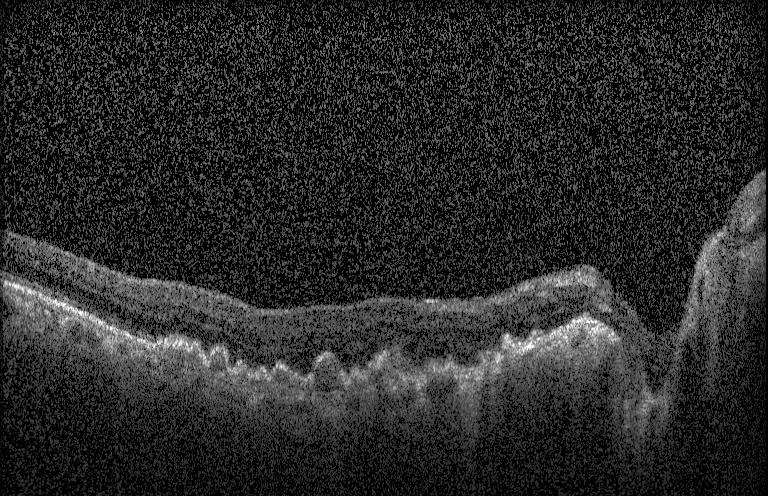

Macular OCT demonstrating choroidal neovascularization.